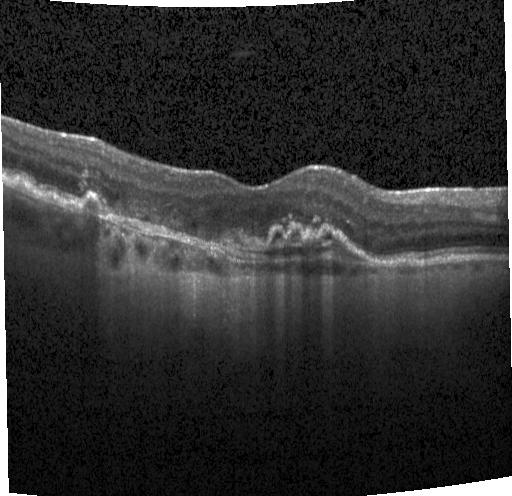 Retinal OCT cross-section.
Assessment: CNV.